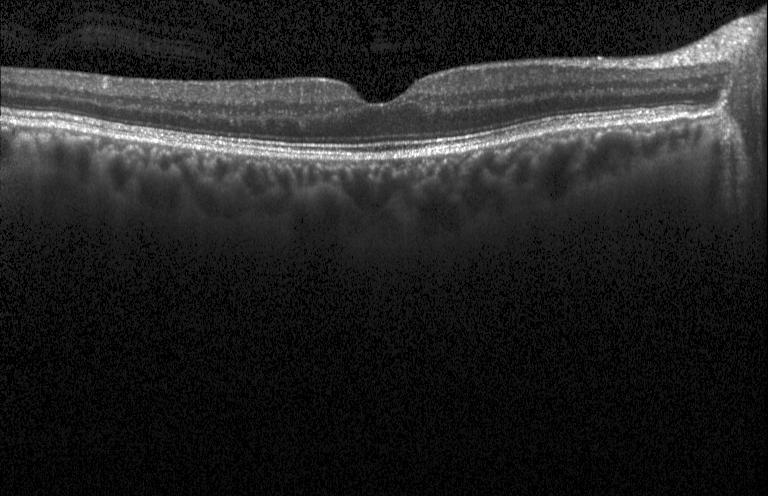

SD-OCT. Centered on the fovea. Retinal OCT B-scan.
Diagnosis: neither choroidal neovascularization, diabetic macular edema, nor drusen.